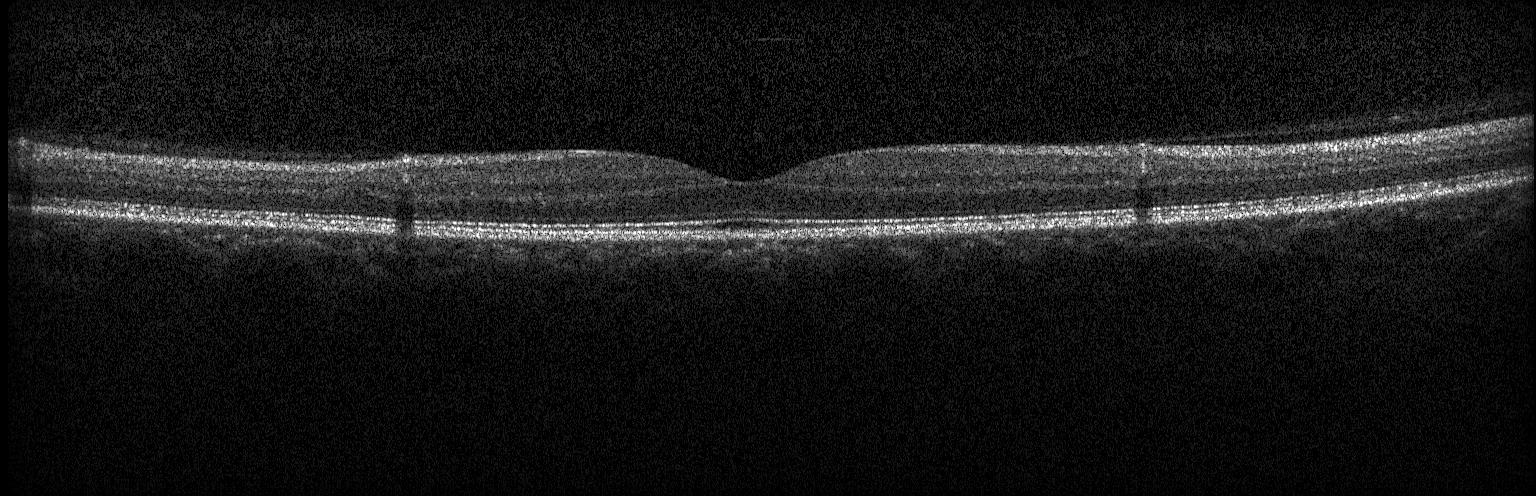

Retinal OCT cross-section · spectral-domain optical coherence tomography
Macular OCT: no choroidal neovascularization, no diabetic macular edema, and no drusen.